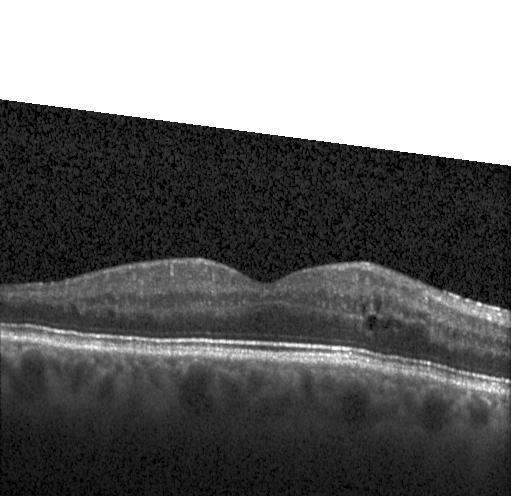

Fovea-centered · spectral-domain OCT · OCT line scan — Finding: diabetic macular edema (DME).